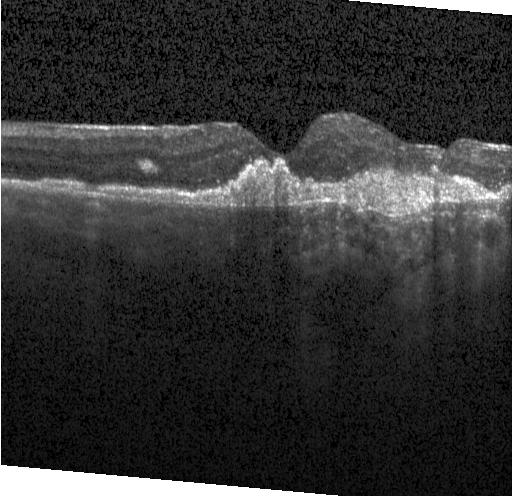 Optical coherence tomography scan. Spectral-domain OCT
Finding: choroidal neovascularization (CNV).